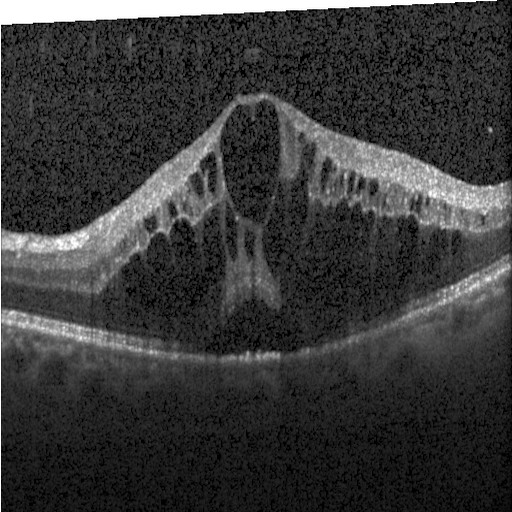

Instrument: Heidelberg Spectralis; retinal OCT B-scan; horizontal scan through the fovea.
Diabetic macular edema (DME).